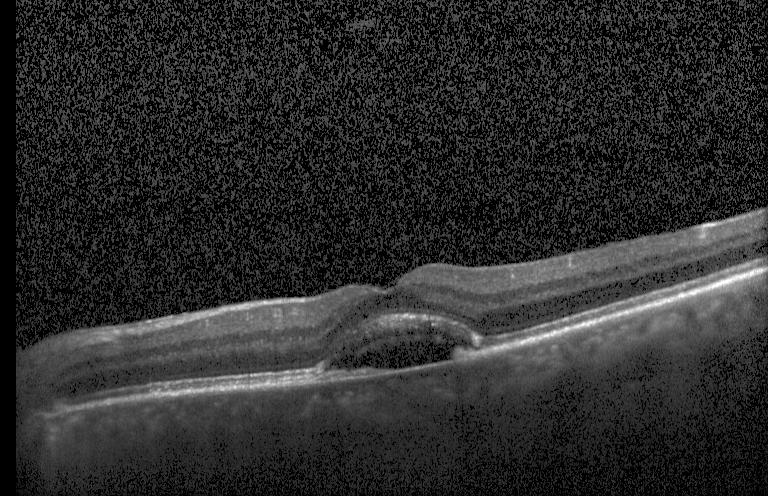
OCT B-scan showing choroidal neovascularization.